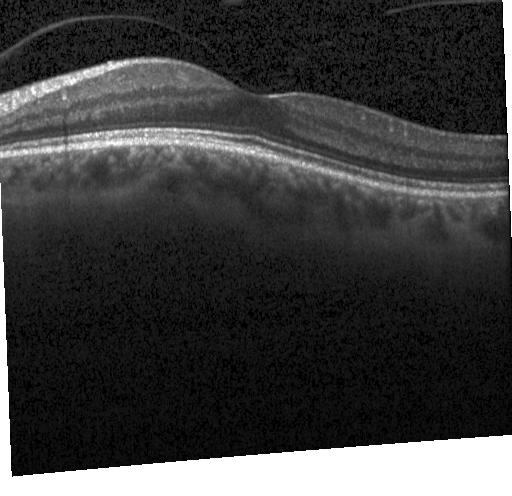
Assessment: no CNV, DME, or drusen.